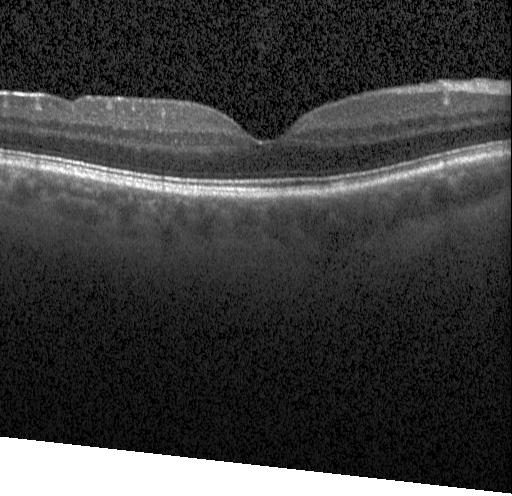

Instrument: Heidelberg Spectralis. Spectral-domain optical coherence tomography. Optical coherence tomography B-scan. Centered on the fovea — Diagnosis: no choroidal neovascularization, no diabetic macular edema, and no drusen.